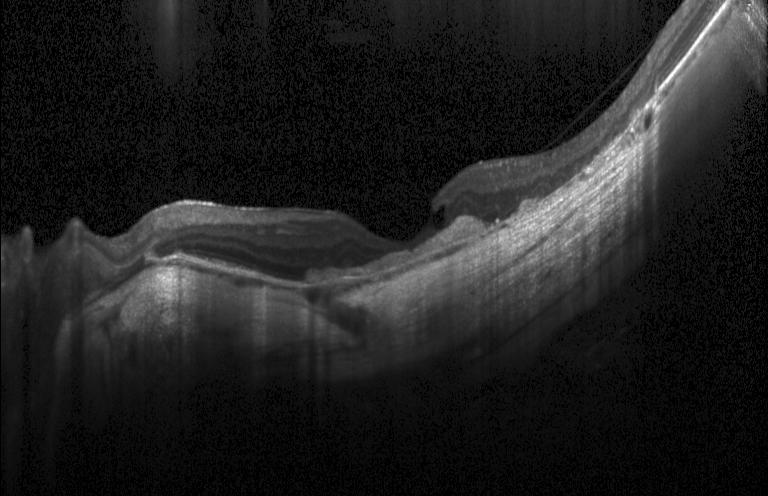

Dx: choroidal neovascularization.